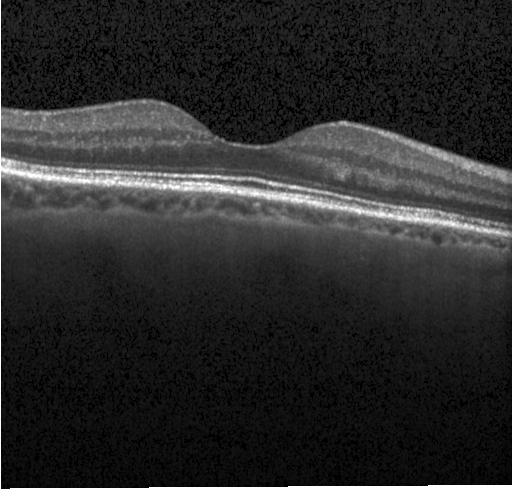
Impression: no CNV, no DME, and no drusen.